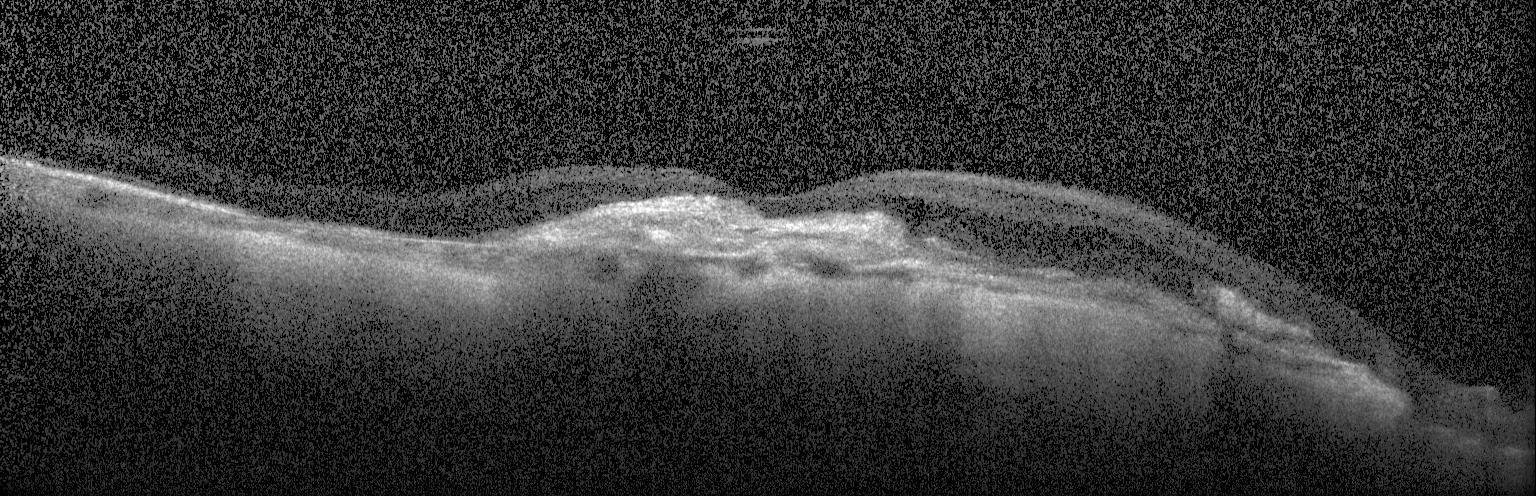
Retinal OCT cross-section; spectral-domain OCT; fovea-centered; acquired on a Heidelberg Spectralis — Dx: a choroidal neovascular membrane.